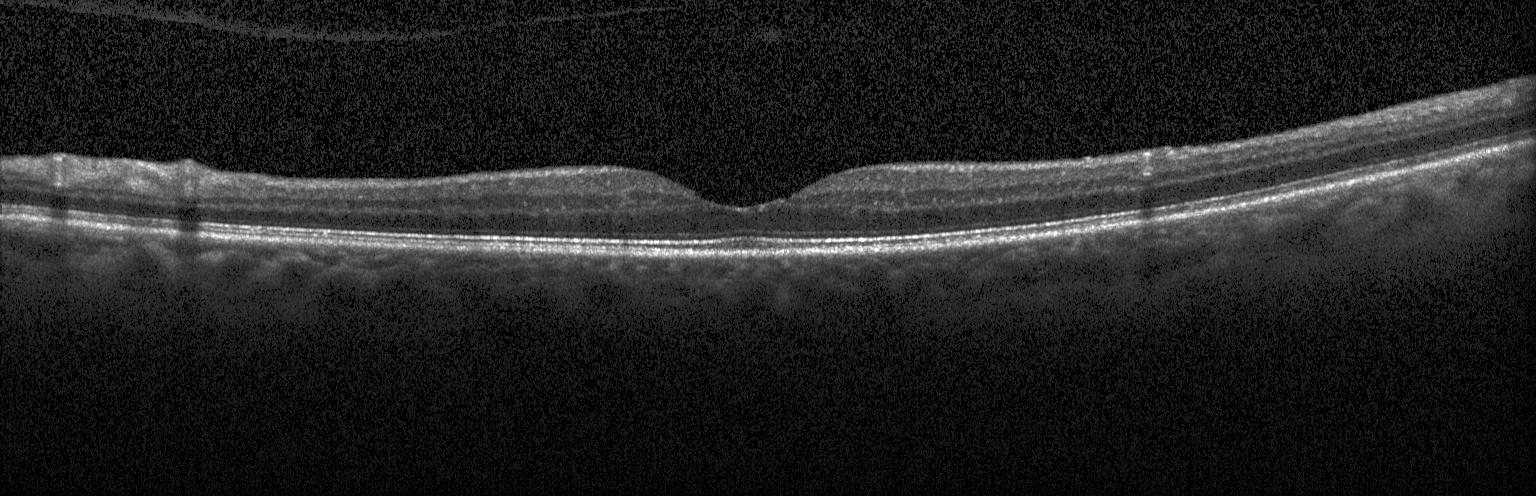

Optical coherence tomography scan — The scan shows no CNV, no DME, and no drusen.